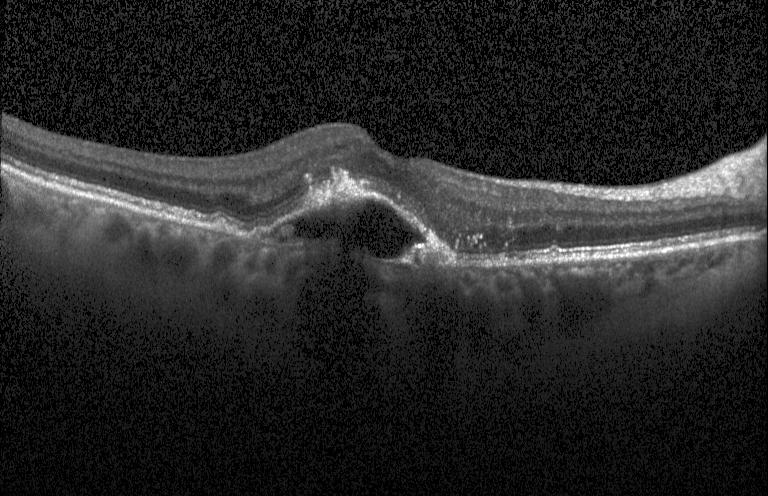

Spectral-domain OCT. OCT B-scan. The scan shows choroidal neovascularization (CNV).